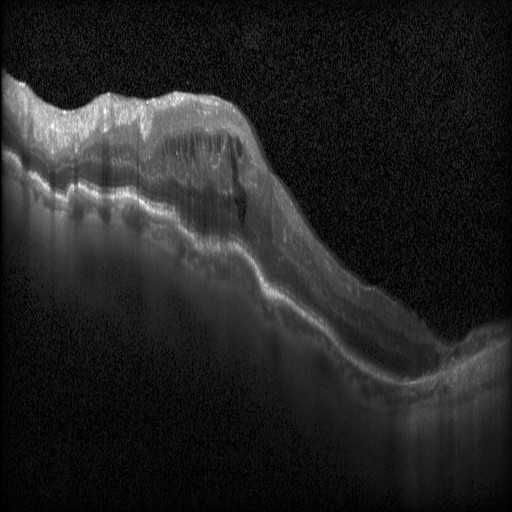 OCT finding: diabetic macular edema.